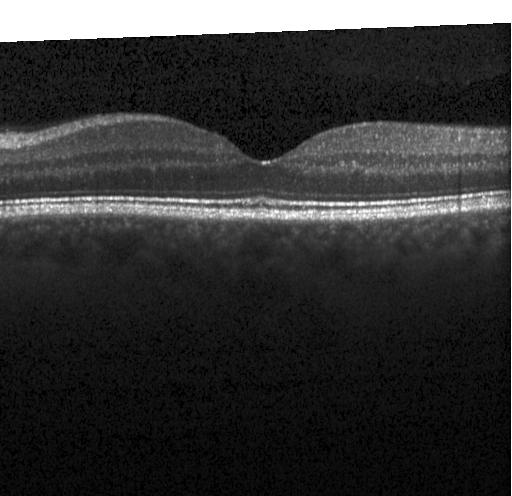

Macular OCT: no evidence of choroidal neovascularization, diabetic macular edema, or drusen.